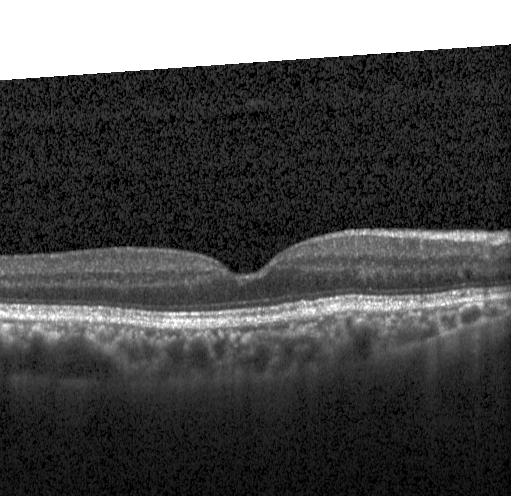
Spectral-domain OCT B-scan: no evidence of choroidal neovascularization, diabetic macular edema, or drusen.